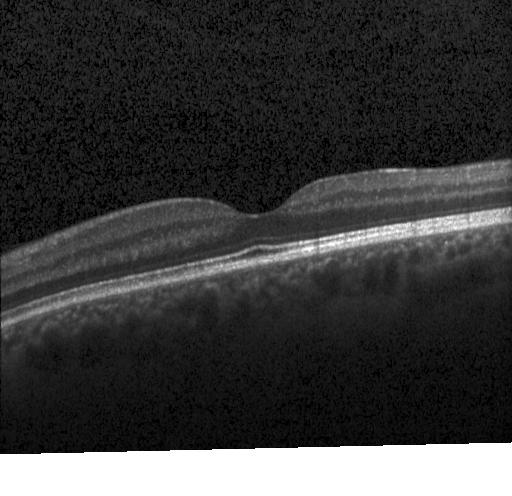

OCT B-scan showing neither CNV, DME, nor drusen.